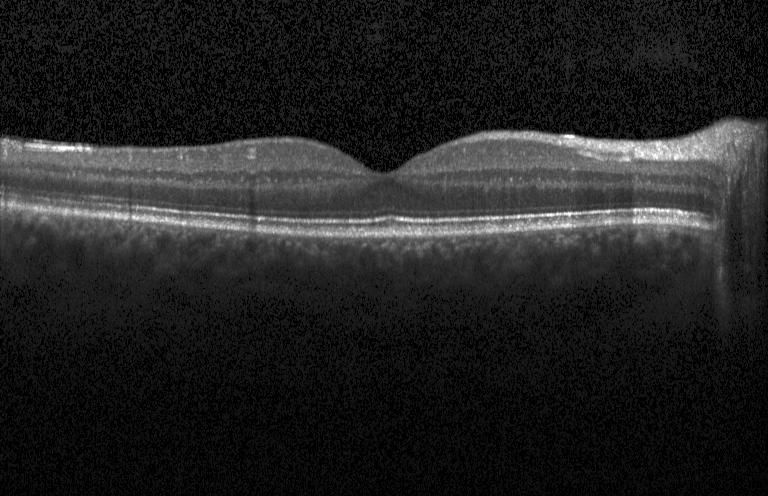 Acquired on a Heidelberg Spectralis. OCT line scan. Diagnosis: no choroidal neovascularization, no diabetic macular edema, and no drusen.